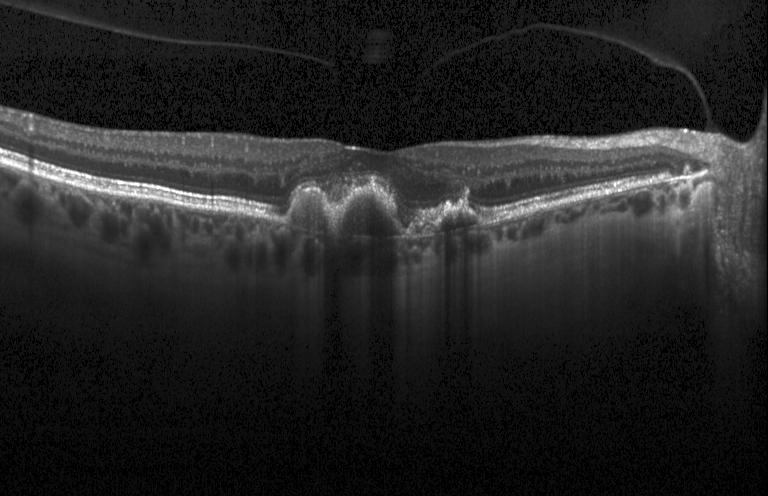 Instrument: Heidelberg Spectralis, SD-OCT, retinal OCT cross-section — Finding: a choroidal neovascular membrane.